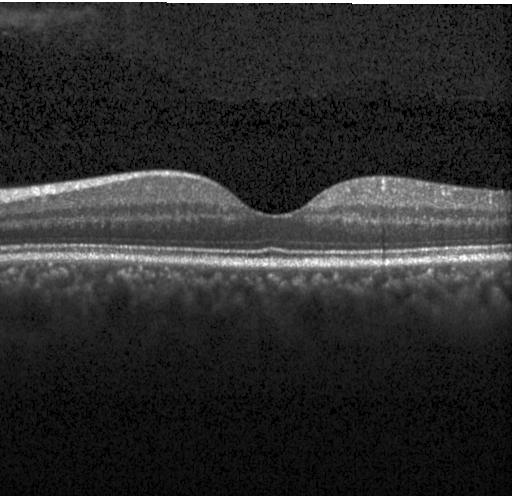

Finding: no CNV, DME, or drusen.